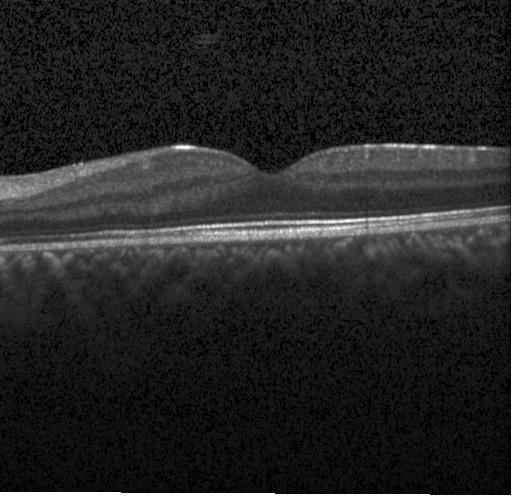

OCT line scan
OCT finding: no evidence of choroidal neovascularization, diabetic macular edema, or drusen.